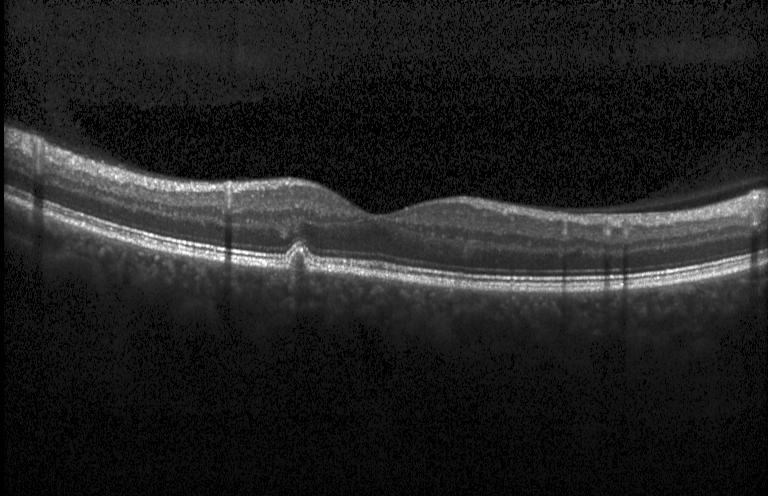

Impression: sub-RPE drusenoid deposits.